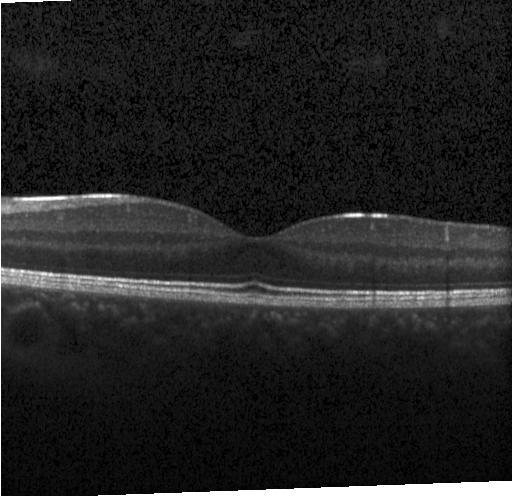 Heidelberg Spectralis OCT system · optical coherence tomography B-scan.
OCT finding: neither choroidal neovascularization, diabetic macular edema, nor drusen.